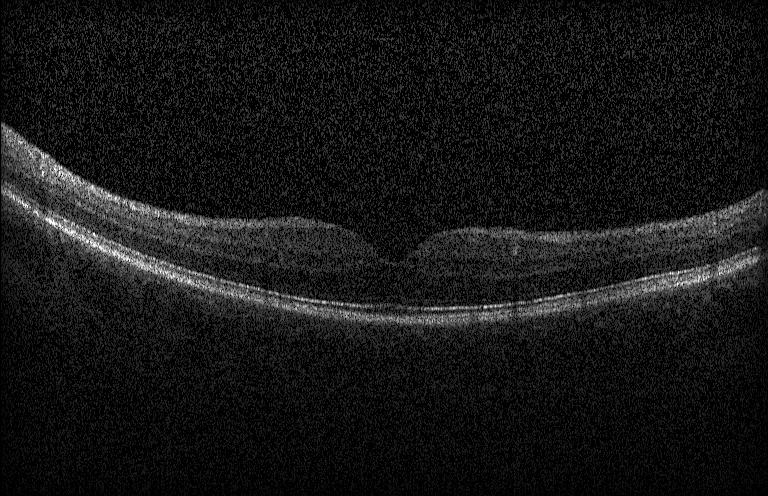

Impression: neither CNV, DME, nor drusen.